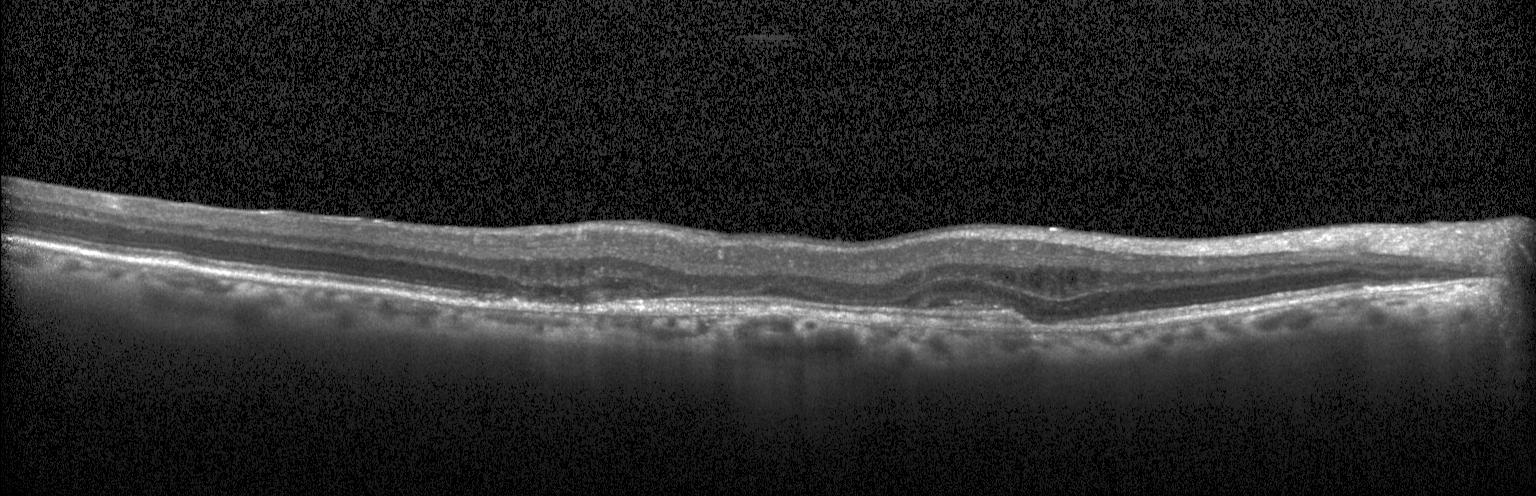
This B-scan demonstrates a choroidal neovascular membrane.